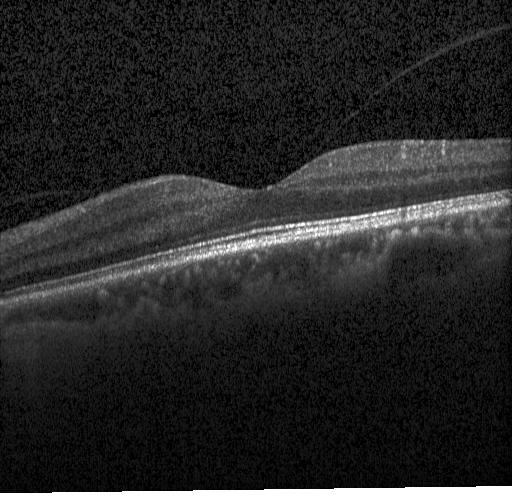
Optical coherence tomography B-scan.
Assessment: no CNV, DME, or drusen.